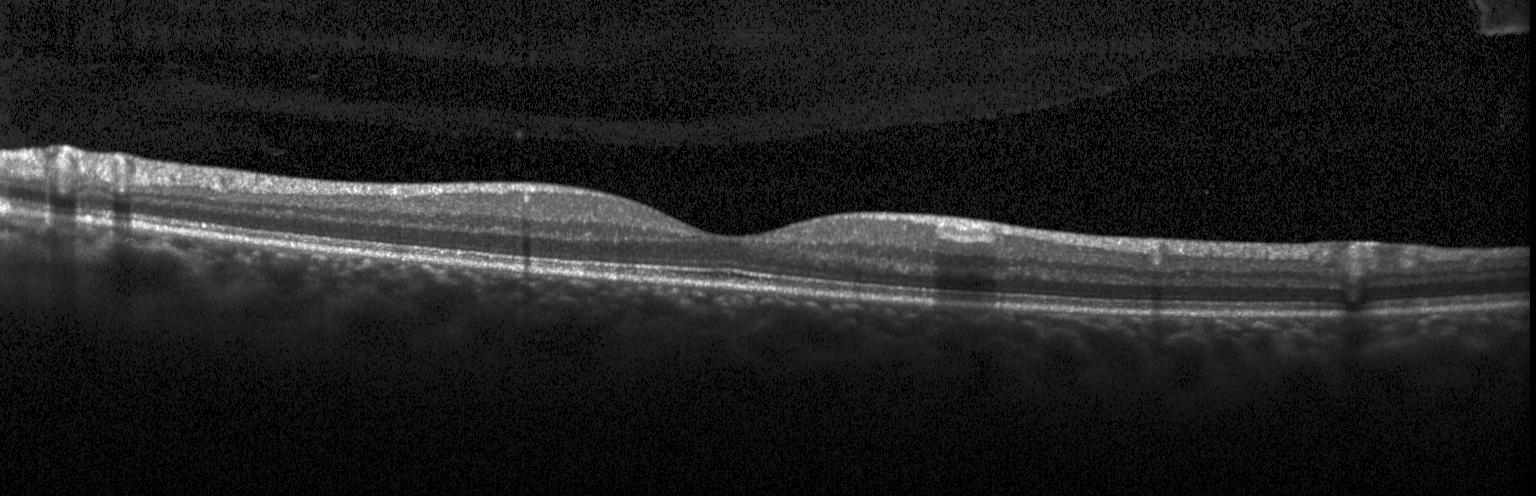

Macular scan. Instrument: Heidelberg Spectralis. Spectral-domain optical coherence tomography. Retinal OCT cross-section. Impression: no choroidal neovascularization, diabetic macular edema, or drusen.